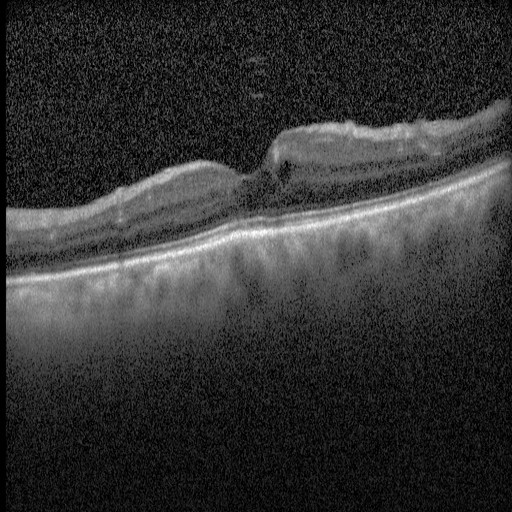
Diabetic macular edema.